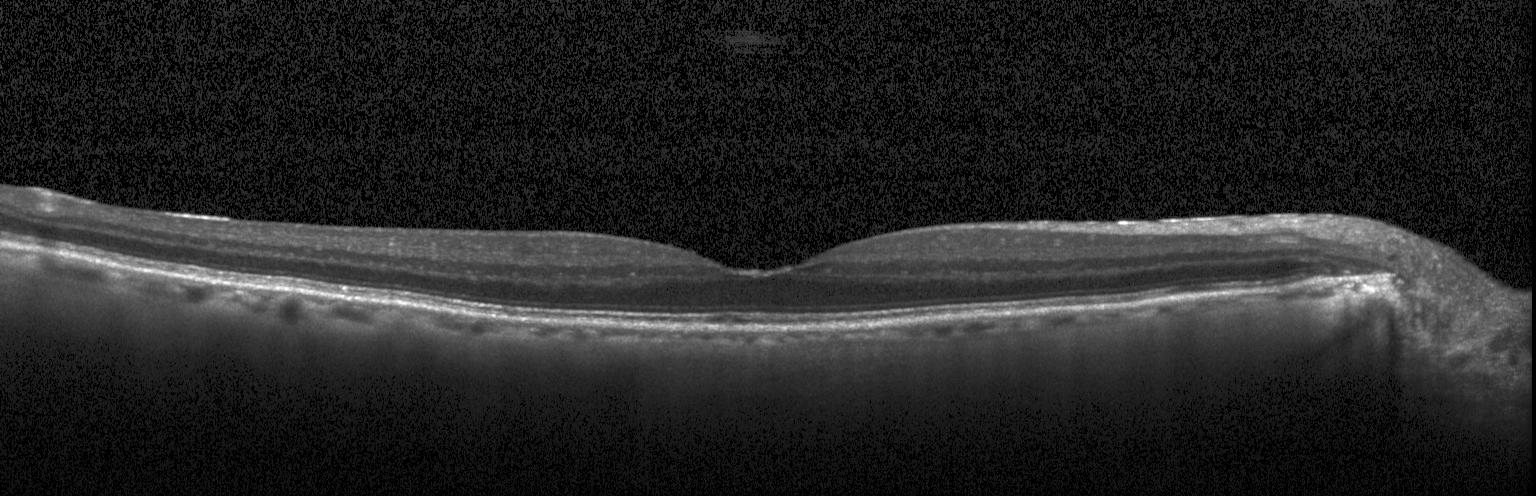
Assessment: neither CNV, DME, nor drusen.